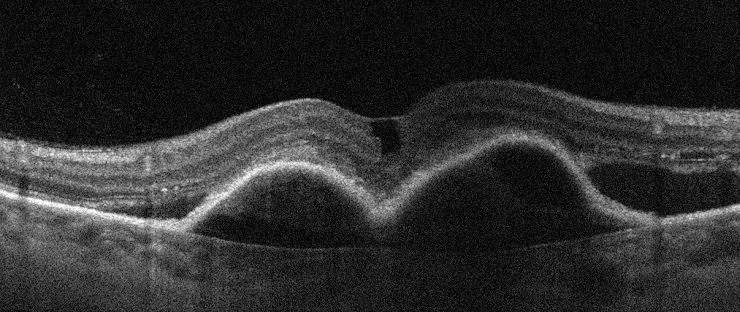

Instrument: Optovue Avanti RTVue XR. Through the macula. OCT line scan.
Diagnosis: AMD.